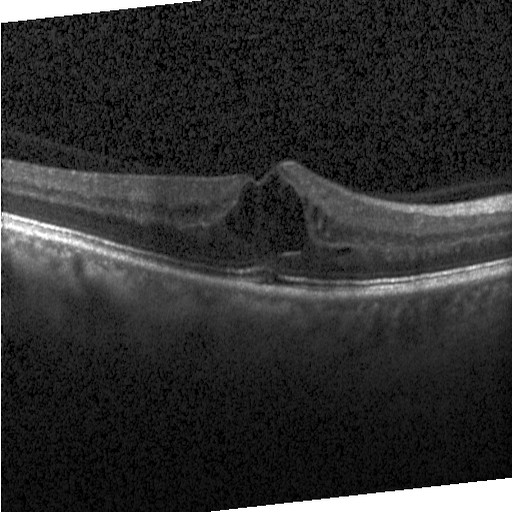

OCT finding: diabetic macular edema (DME).